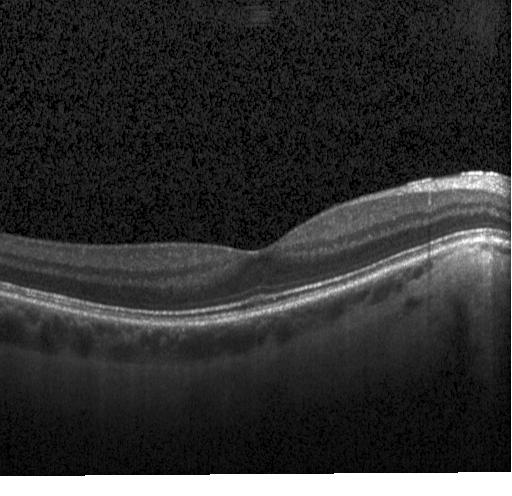 The scan shows no evidence of choroidal neovascularization, diabetic macular edema, or drusen.